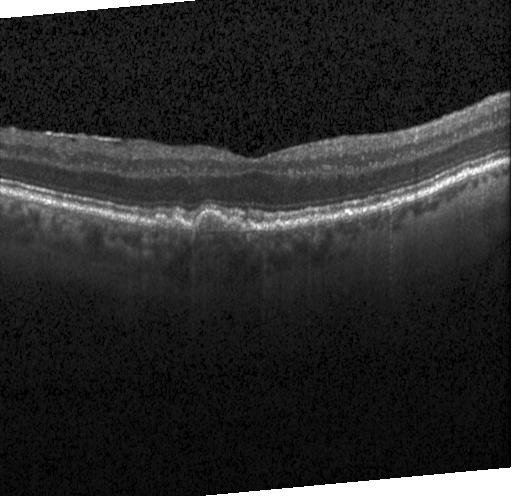

SD-OCT. Retinal OCT cross-section. Through the macula. Heidelberg Spectralis OCT system
Dx: drusen.